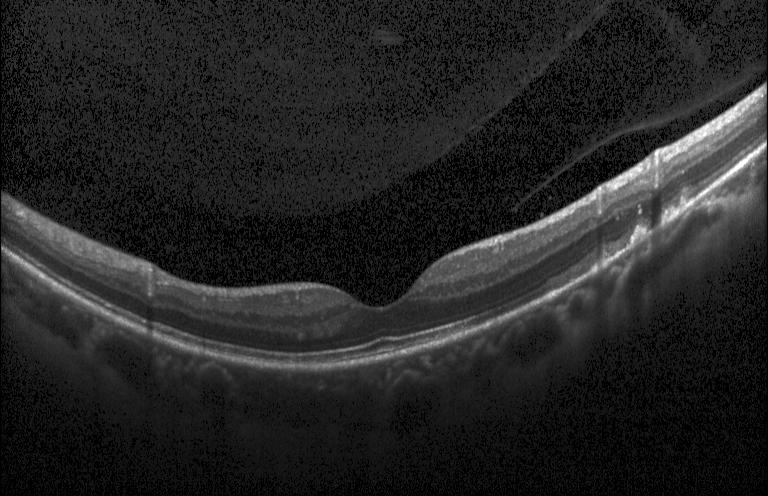

Retinal OCT cross-section. This B-scan demonstrates drusen.